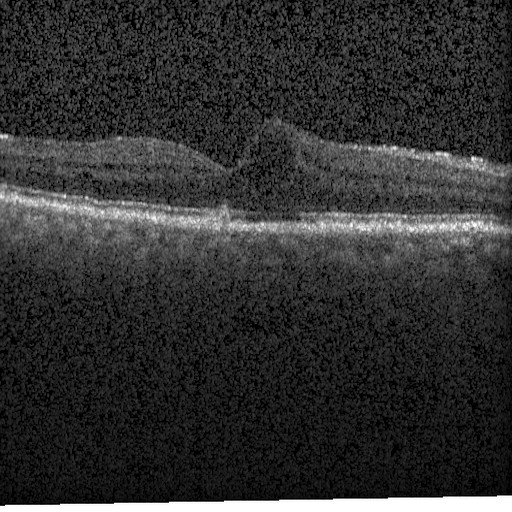

Diabetic macular edema (DME).